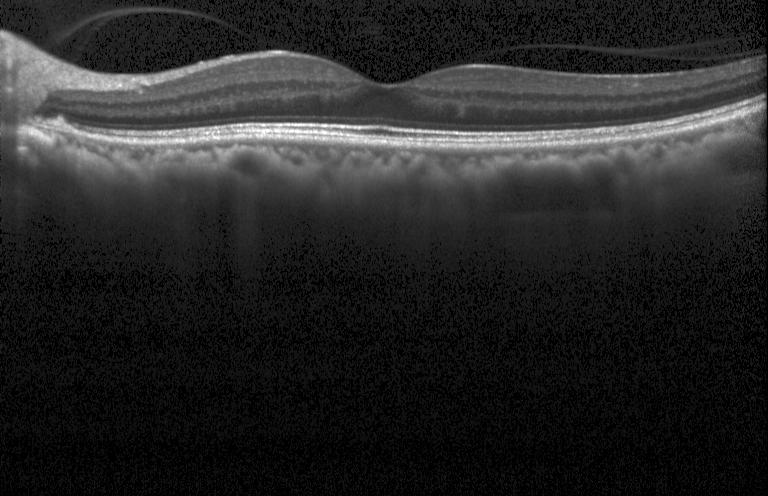
Retinal OCT cross-section — Finding: neither CNV, DME, nor drusen.